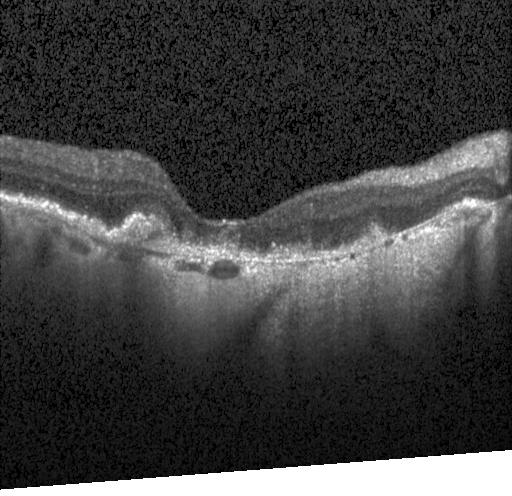
Retinal OCT cross-section, Heidelberg Spectralis OCT system, through the macula, SD-OCT. Dx: a choroidal neovascular membrane.